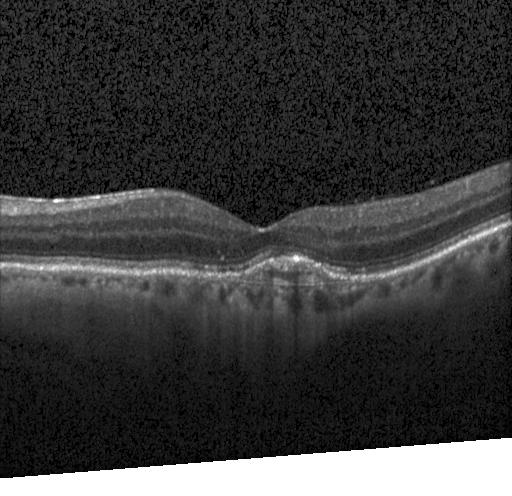 Optical coherence tomography scan · acquired on a Heidelberg Spectralis · SD-OCT · through the macula
Diagnosis: a choroidal neovascular membrane.